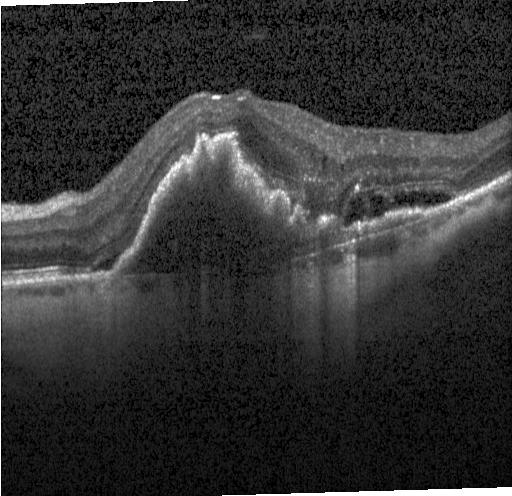
Impression: CNV.